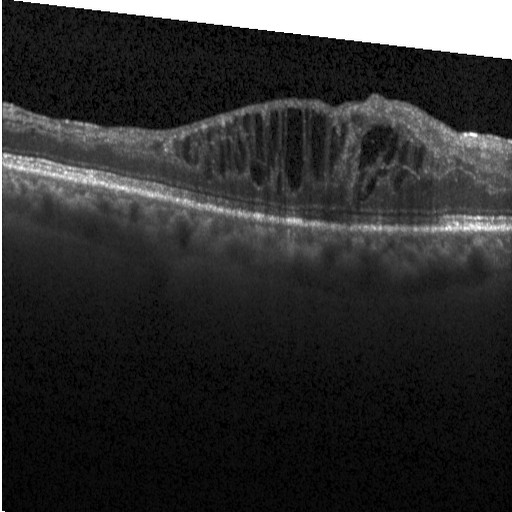

Instrument: Heidelberg Spectralis; retinal OCT B-scan; macular scan; SD-OCT — Macular OCT: diabetic macular edema.